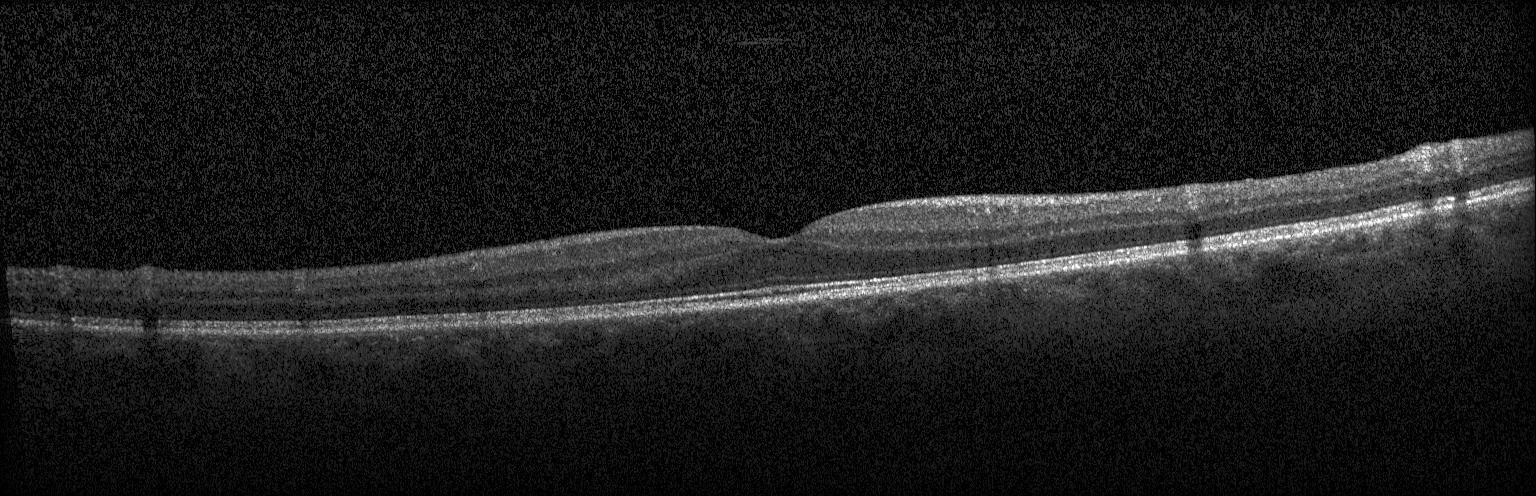
Spectral-domain OCT; OCT line scan
The scan shows no evidence of choroidal neovascularization, diabetic macular edema, or drusen.